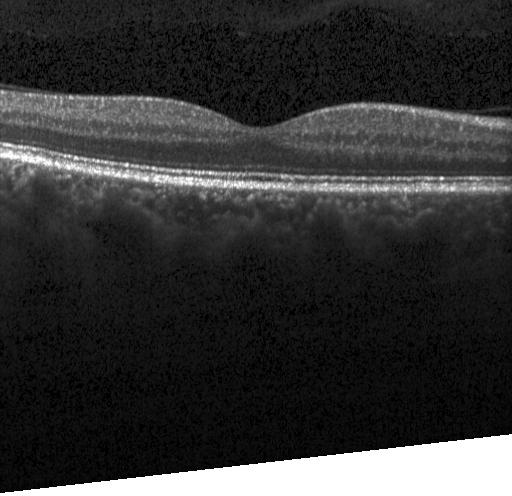

Macular OCT demonstrating no evidence of choroidal neovascularization, diabetic macular edema, or drusen.